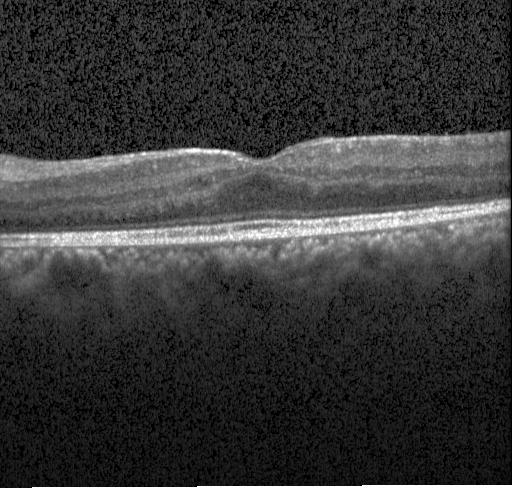 SD-OCT; fovea-centered; retinal OCT B-scan. Assessment: diabetic macular edema.